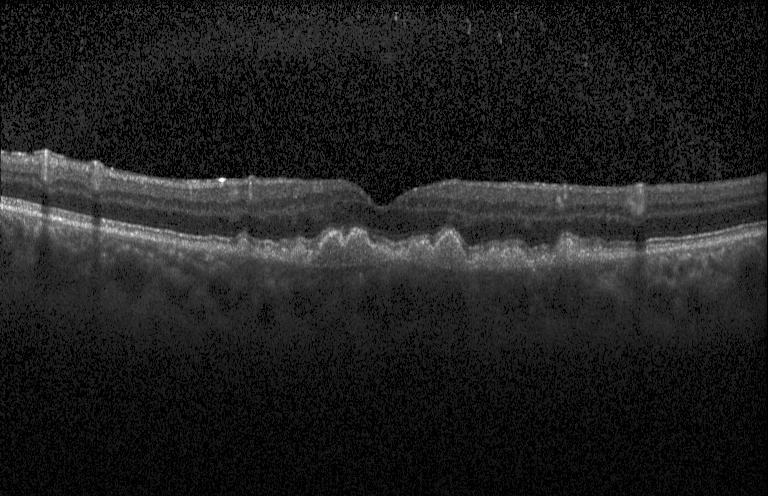
Spectral-domain OCT, centered on the fovea, OCT line scan, Heidelberg Spectralis.
Finding: choroidal neovascularization (CNV).